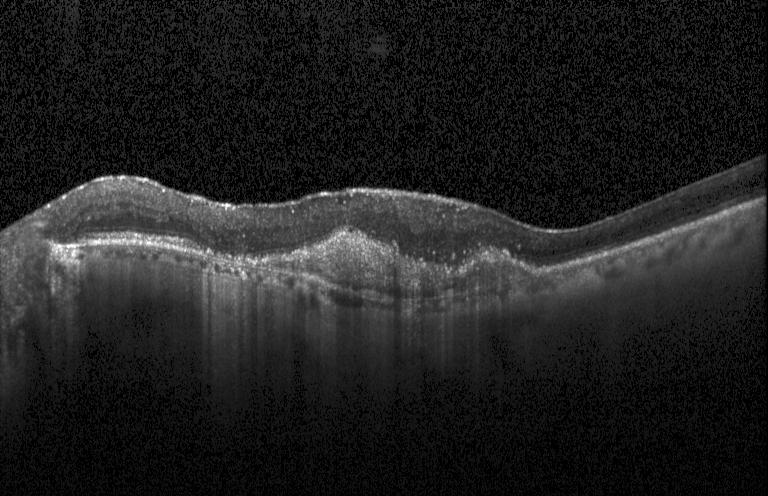
Choroidal neovascularization.